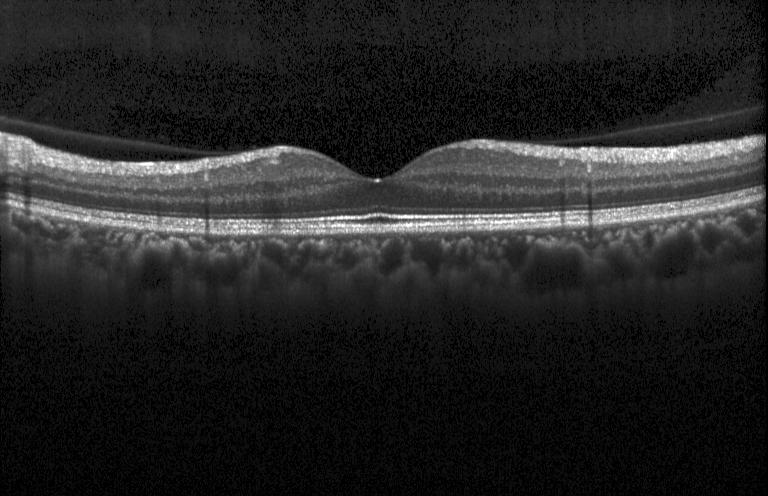
Macular scan; optical coherence tomography B-scan; Heidelberg Spectralis — Macular OCT: neither choroidal neovascularization, diabetic macular edema, nor drusen.